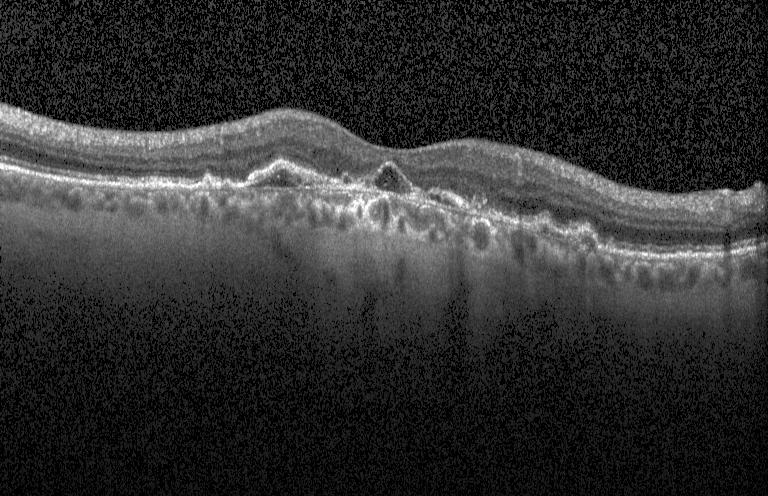 Acquired on a Heidelberg Spectralis, OCT B-scan. Dx: a choroidal neovascular membrane.